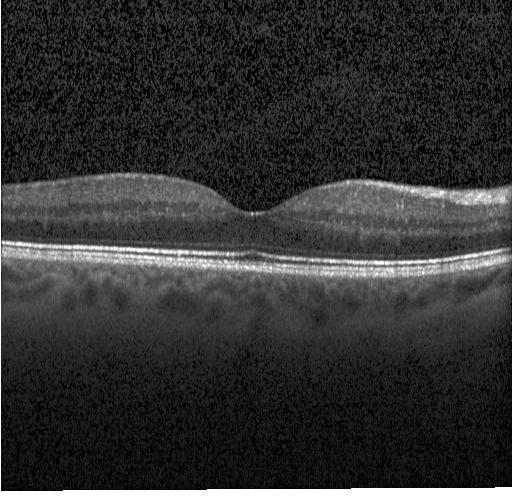 Retinal OCT cross-section showing no choroidal neovascularization, diabetic macular edema, or drusen.